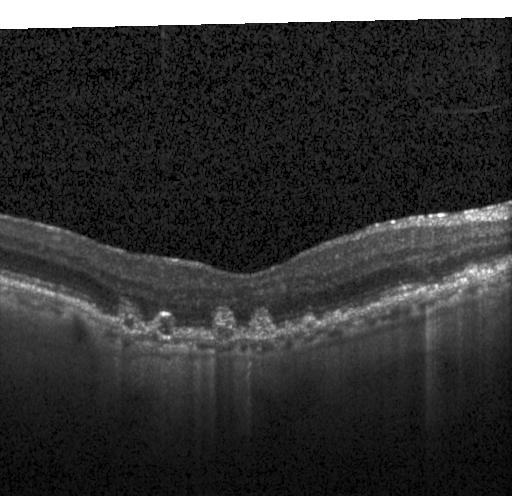

OCT B-scan. Spectral-domain OCT.
Diagnosis: choroidal neovascularization.